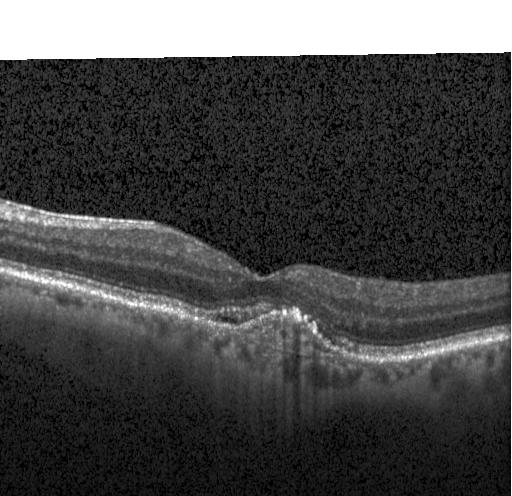 Macular scan. OCT B-scan. Instrument: Heidelberg Spectralis. Spectral-domain optical coherence tomography
Macular OCT: a choroidal neovascular membrane.